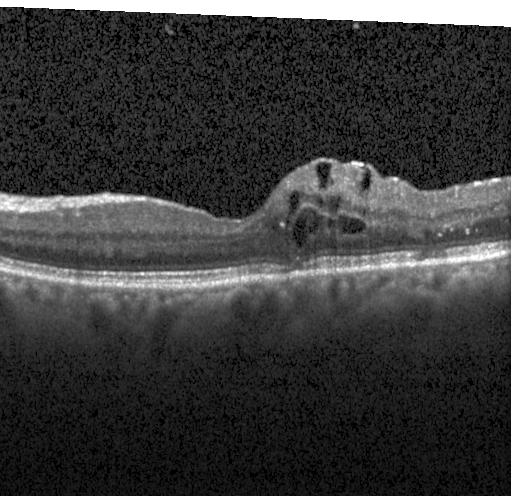
Diagnosis: diabetic macular edema.